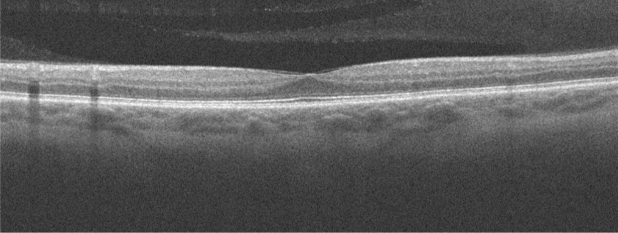

Retinal OCT B-scan · instrument: Optovue Avanti RTVue XR. Impression: no AMD, DME, ERM, RAO, RVO, or VID.